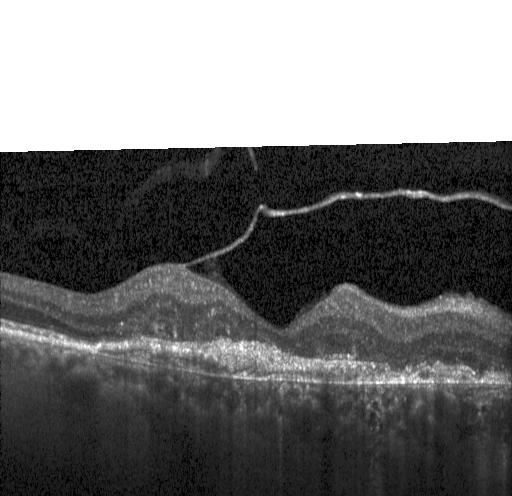

Macular OCT demonstrating choroidal neovascularization (CNV).